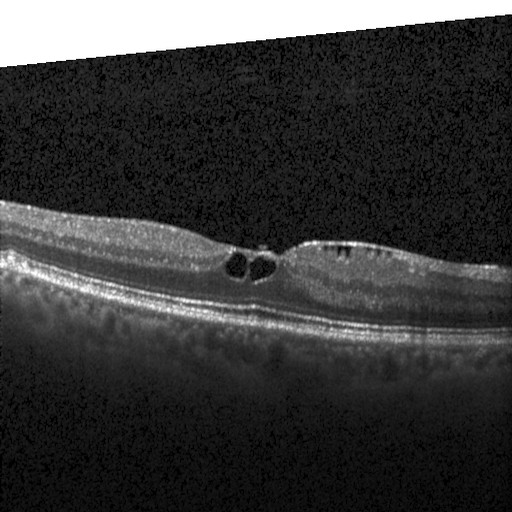
OCT B-scan — Assessment: diabetic macular edema.